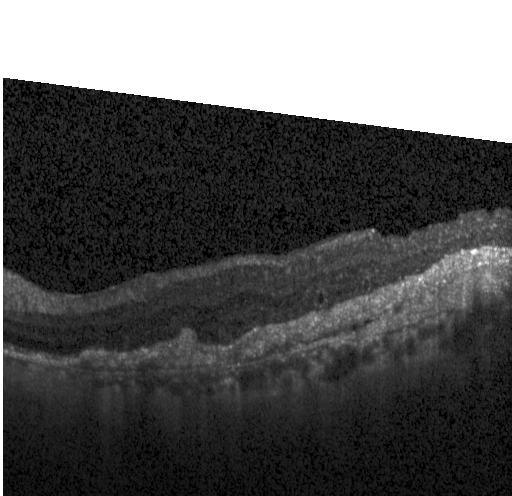

Fovea-centered · Heidelberg Spectralis · retinal OCT B-scan
Assessment: choroidal neovascularization.